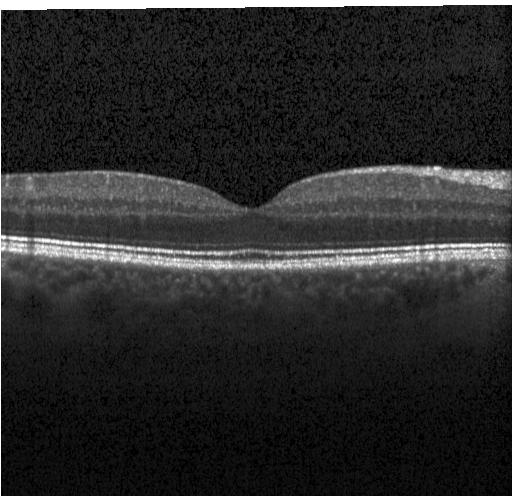

Macular OCT demonstrating no CNV, DME, or drusen.